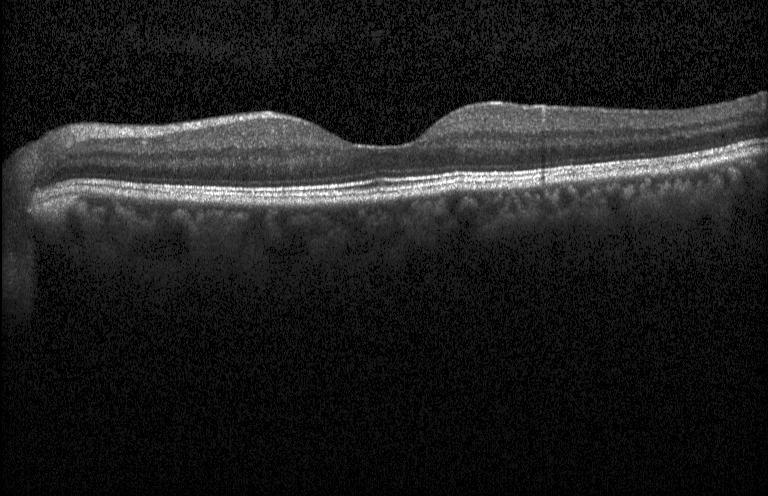
Spectral-domain OCT, optical coherence tomography scan, Heidelberg Spectralis, fovea-centered — Dx: neither choroidal neovascularization, diabetic macular edema, nor drusen.